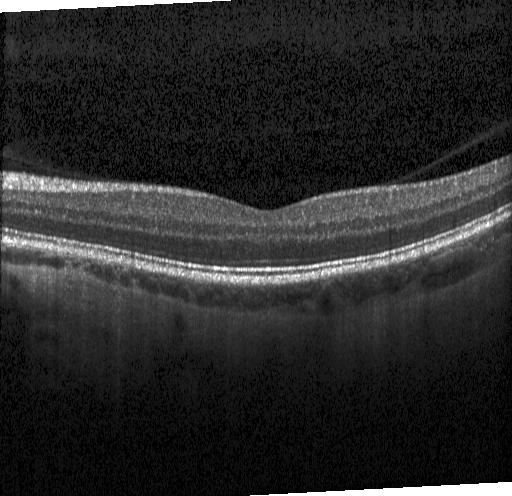

OCT B-scan.
This B-scan demonstrates neither CNV, DME, nor drusen.